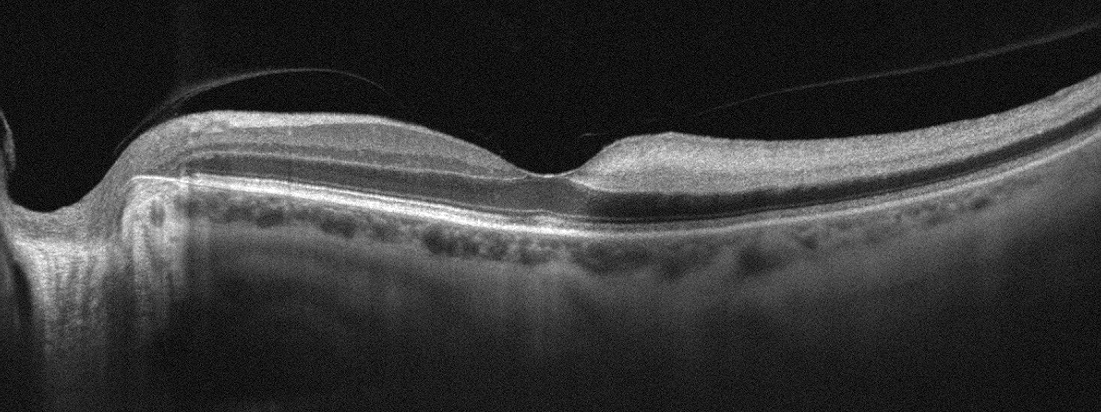 Retinal OCT B-scan.
Impression: retinal artery occlusion (RAO).